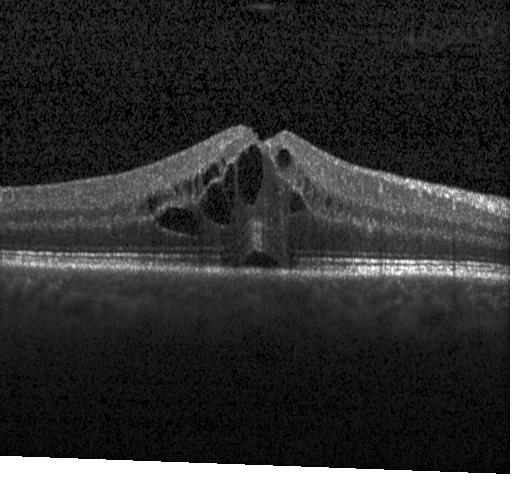 Acquired on a Heidelberg Spectralis · OCT line scan · spectral-domain optical coherence tomography — Finding: diabetic macular edema.